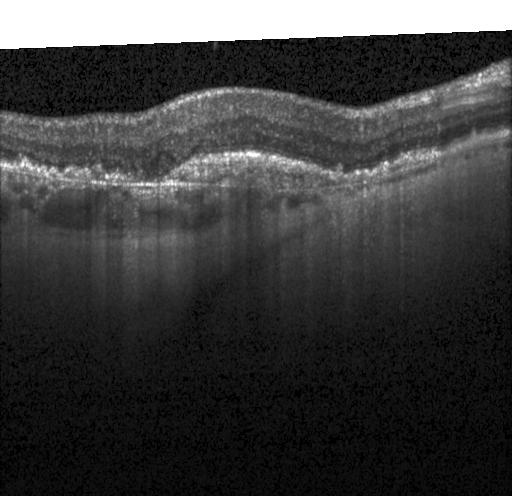

Finding: a choroidal neovascular membrane.